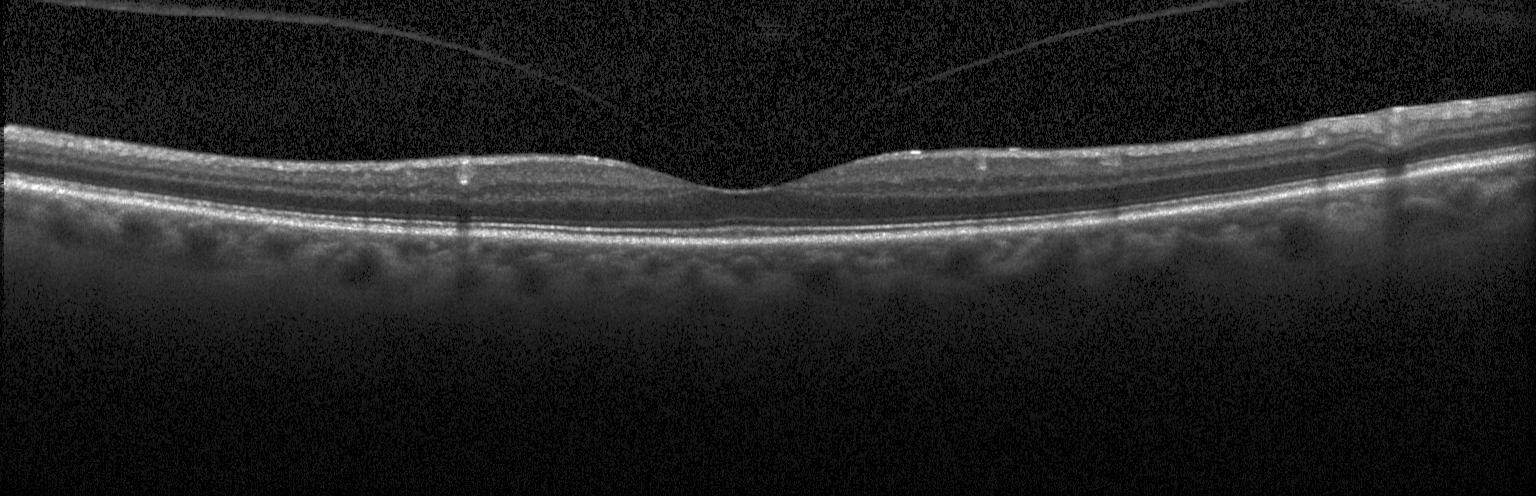

Impression: neither CNV, DME, nor drusen.